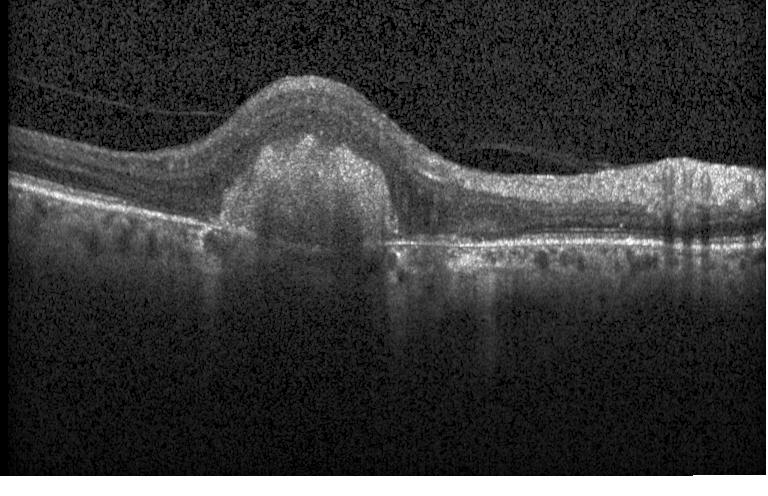 Acquired on a Heidelberg Spectralis; spectral-domain optical coherence tomography; OCT line scan. Impression: a choroidal neovascular membrane.